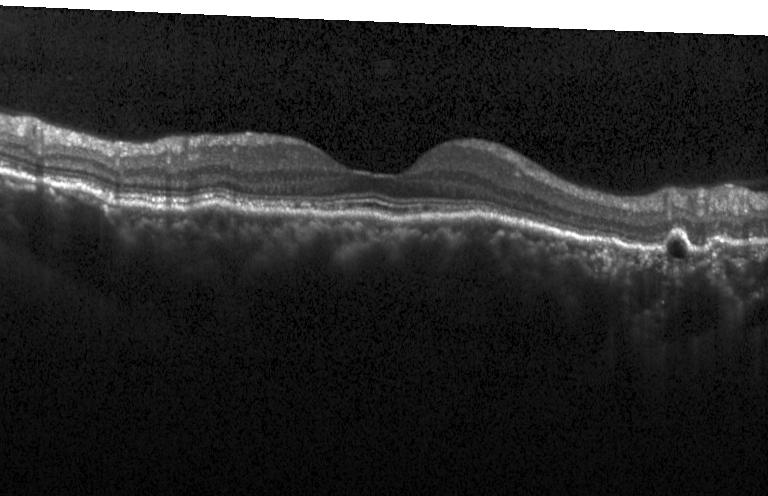

Optical coherence tomography scan — The scan shows CNV.